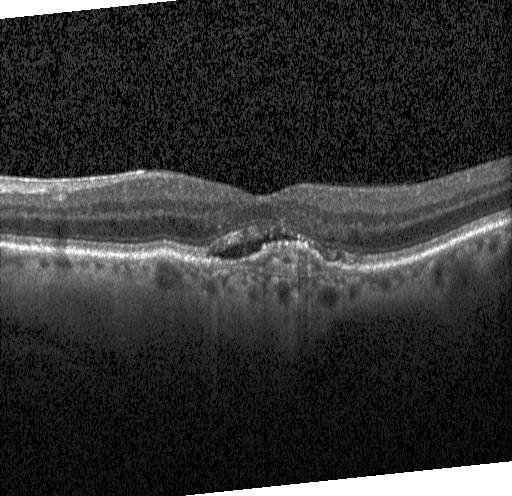

OCT line scan, fovea-centered. Finding: CNV.